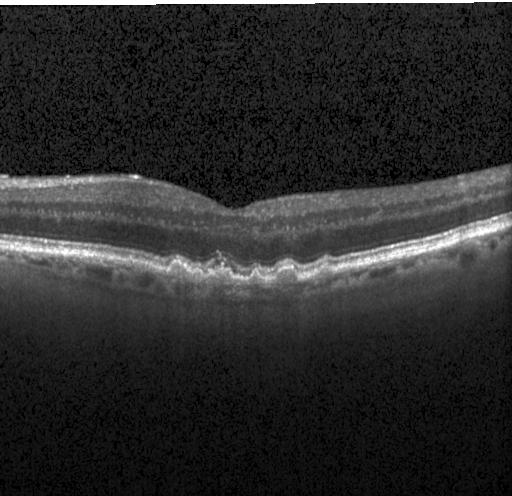
SD-OCT, centered on the fovea, optical coherence tomography B-scan.
Diagnosis: CNV.